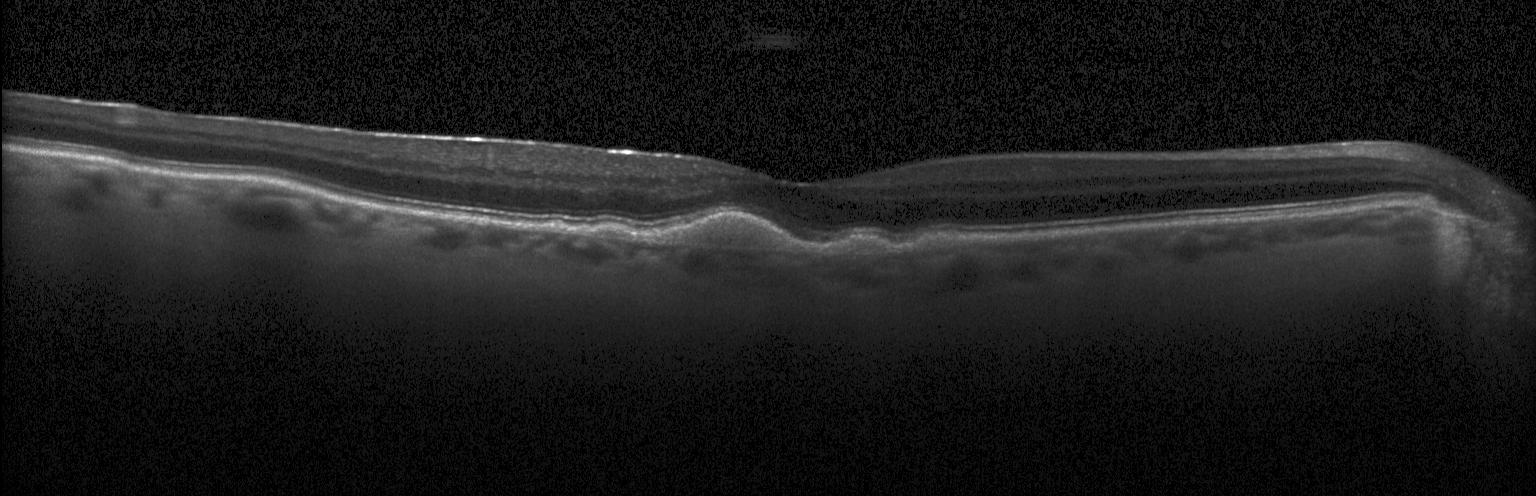 Impression: drusen.